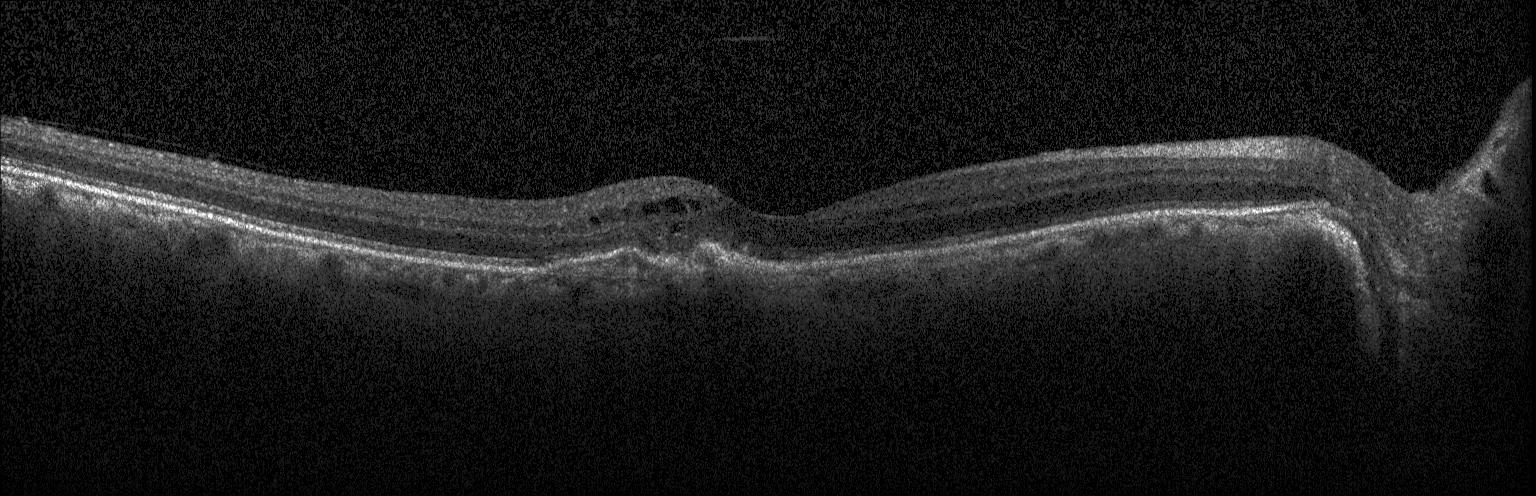 SD-OCT. Retinal OCT cross-section. Impression: a choroidal neovascular membrane.